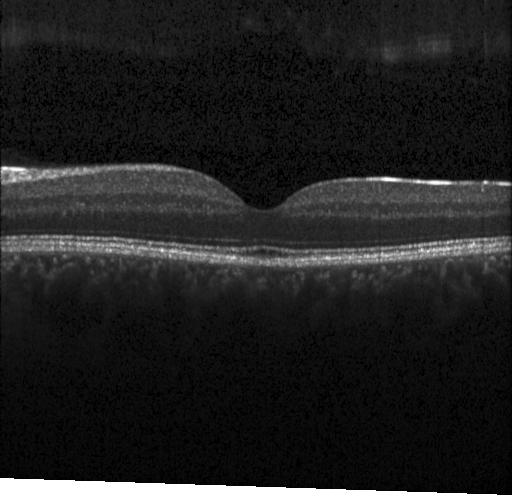 OCT scan showing no CNV, DME, or drusen.